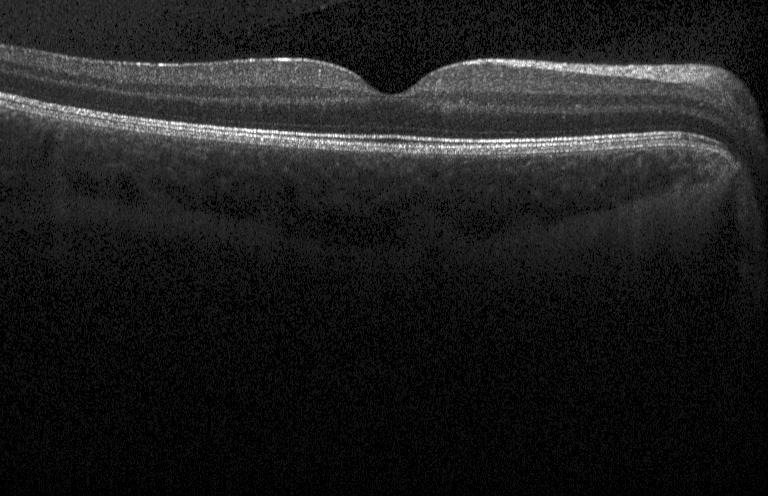
Retinal OCT B-scan, through the macula, spectral-domain optical coherence tomography. Assessment: neither choroidal neovascularization, diabetic macular edema, nor drusen.